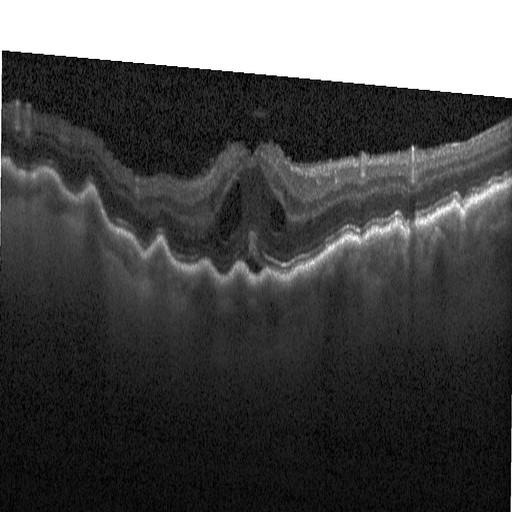
Spectral-domain OCT, retinal OCT cross-section, fovea-centered
Diagnosis: diabetic macular edema (DME).